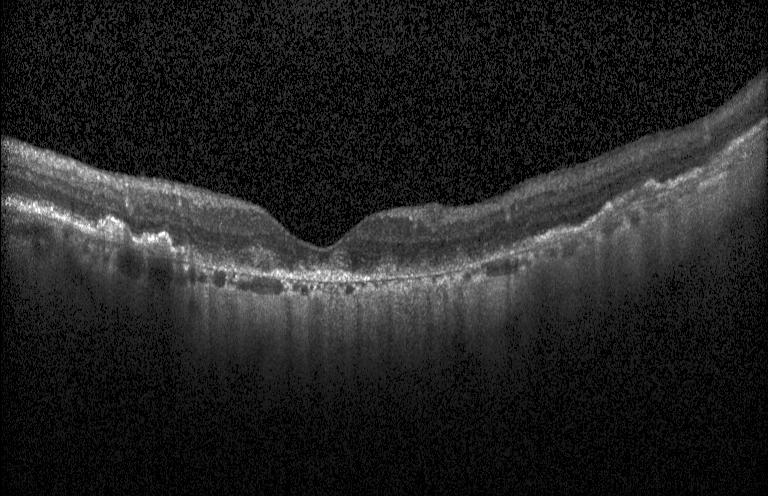 Spectral-domain optical coherence tomography. Heidelberg Spectralis OCT system. OCT line scan. Fovea-centered
This B-scan demonstrates choroidal neovascularization.